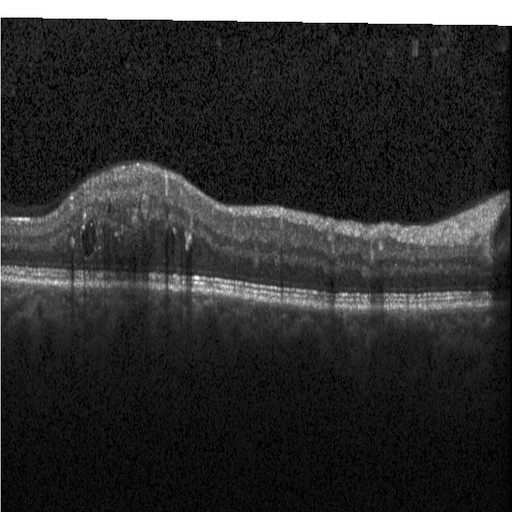 Macular OCT demonstrating DME.